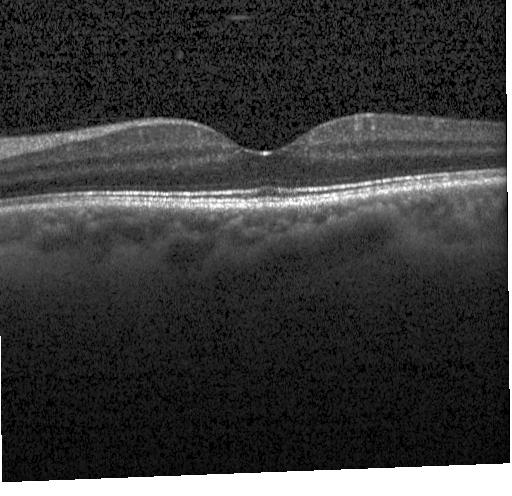 Heidelberg Spectralis. Fovea-centered. Retinal OCT B-scan. Impression: no choroidal neovascularization, no diabetic macular edema, and no drusen.